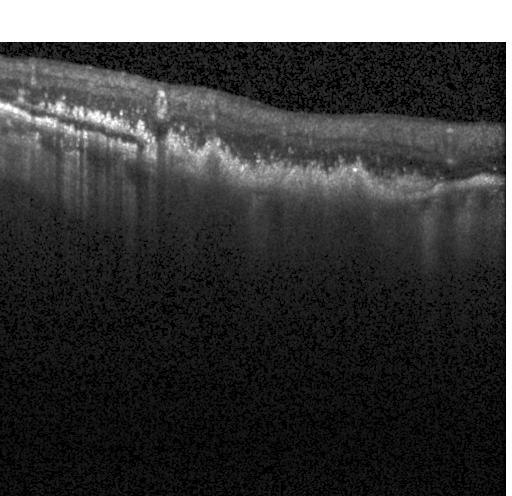 Macular OCT: choroidal neovascularization (CNV).